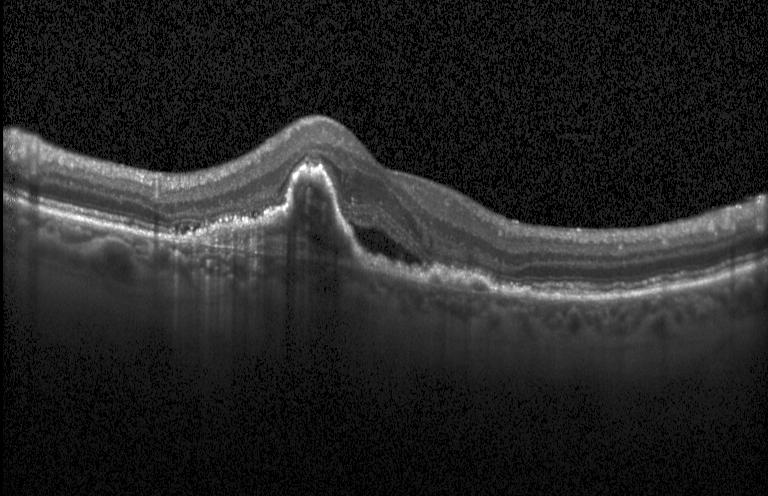
Optical coherence tomography scan · spectral-domain optical coherence tomography — Choroidal neovascularization.